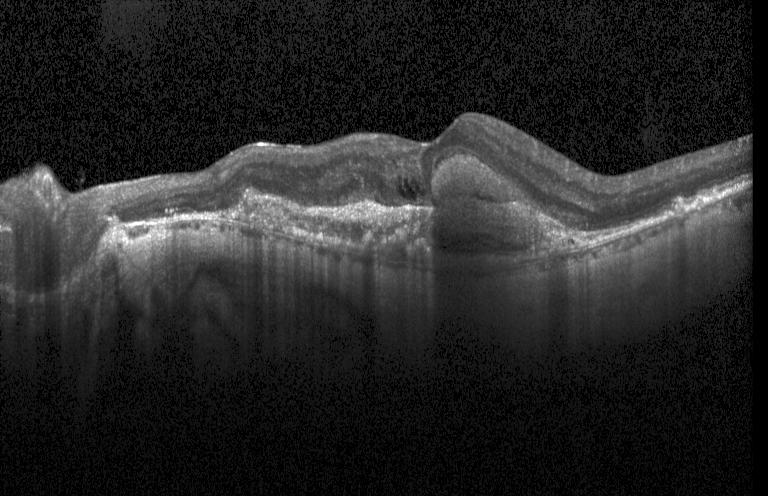
OCT finding: a choroidal neovascular membrane.